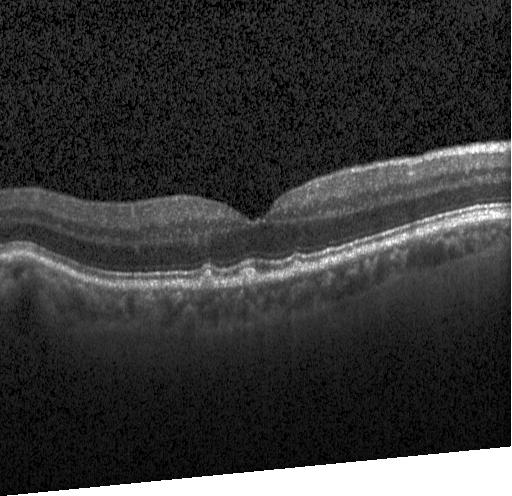

Retinal OCT B-scan, acquired on a Heidelberg Spectralis, horizontal scan through the fovea — Impression: multiple drusen.